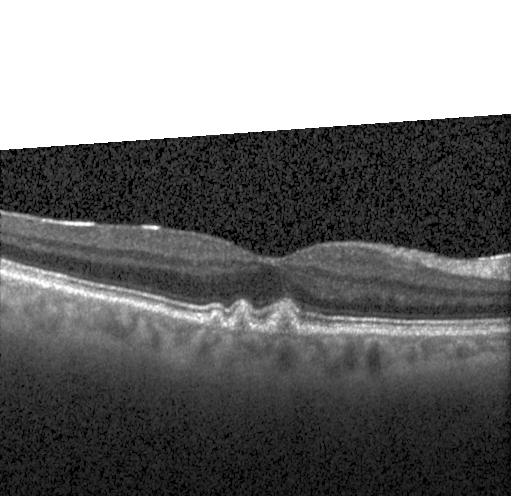

OCT scan showing multiple drusen.